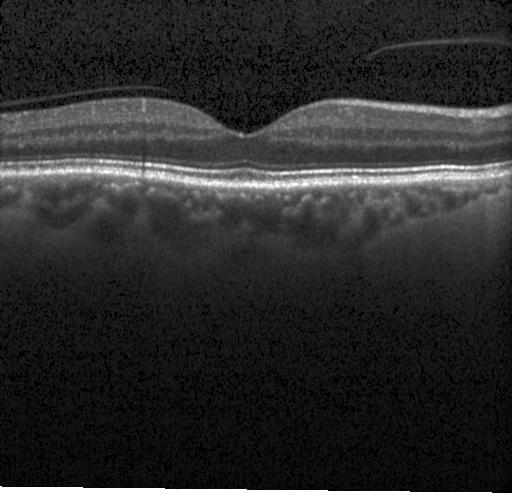

Retinal OCT cross-section. SD-OCT. Heidelberg Spectralis OCT system. Diagnosis: no evidence of choroidal neovascularization, diabetic macular edema, or drusen.